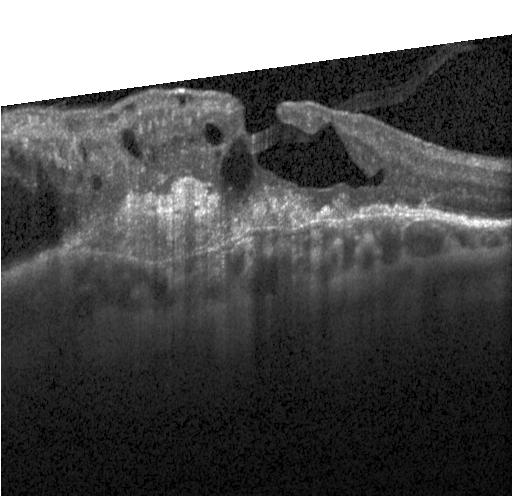

OCT B-scan.
Diagnosis: a choroidal neovascular membrane.